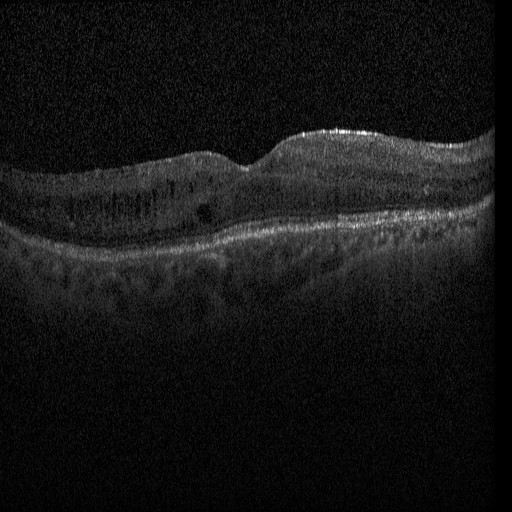 Macular OCT: DME.